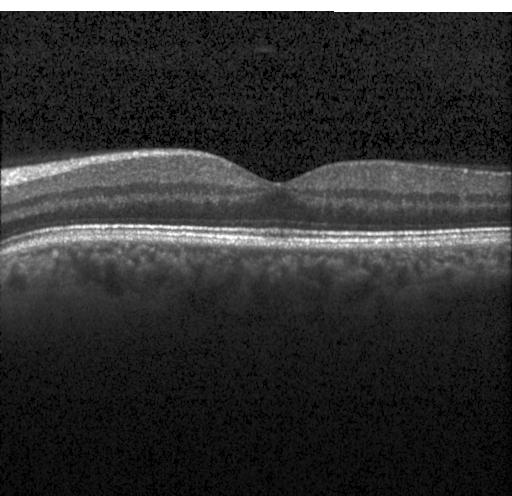
OCT line scan — Impression: no evidence of choroidal neovascularization, diabetic macular edema, or drusen.